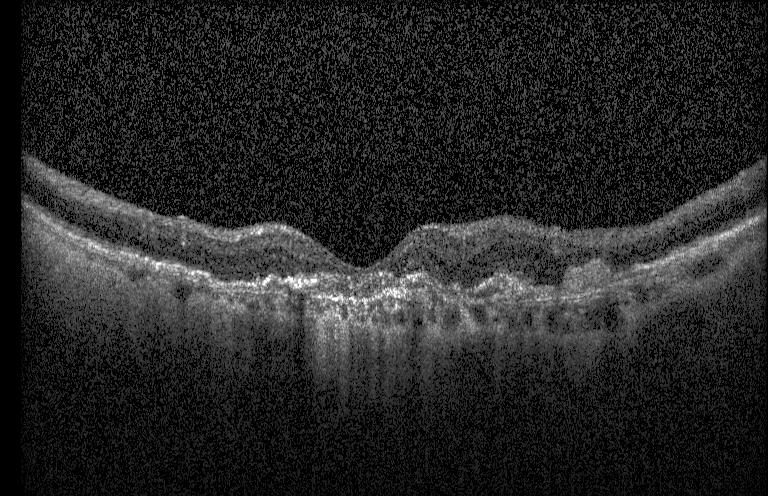

Macular scan, OCT line scan, spectral-domain OCT, acquired on a Heidelberg Spectralis
The scan shows CNV.